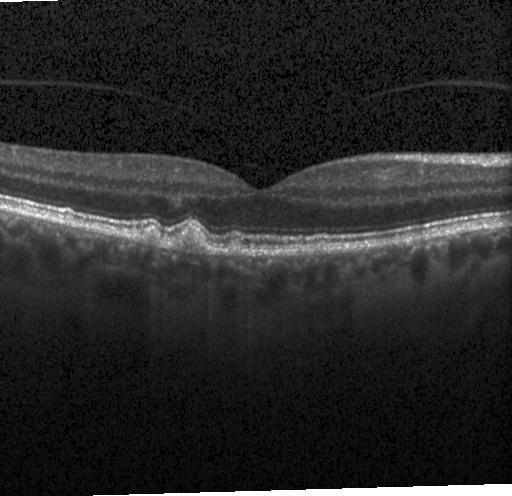 Instrument: Heidelberg Spectralis · optical coherence tomography scan · spectral-domain optical coherence tomography · through the macula. Impression: drusen.